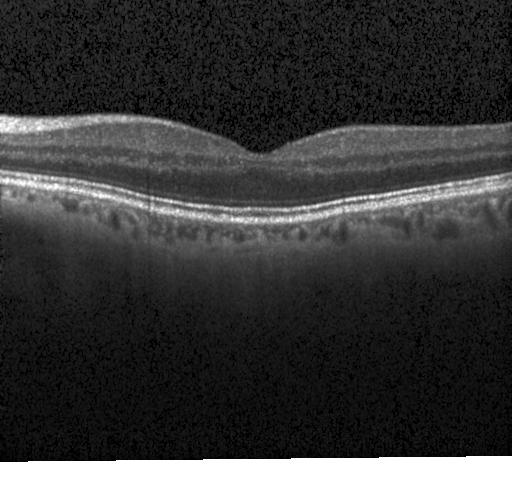

Retinal OCT B-scan
This B-scan demonstrates no evidence of choroidal neovascularization, diabetic macular edema, or drusen.